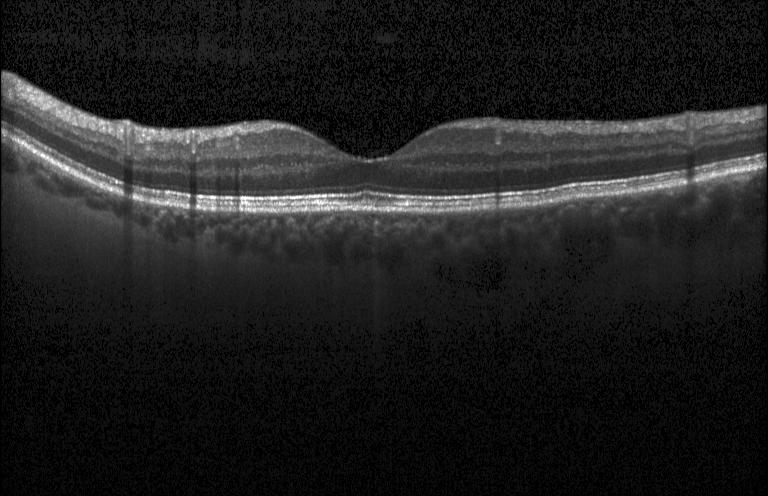

Retinal OCT cross-section — Finding: no choroidal neovascularization, diabetic macular edema, or drusen.